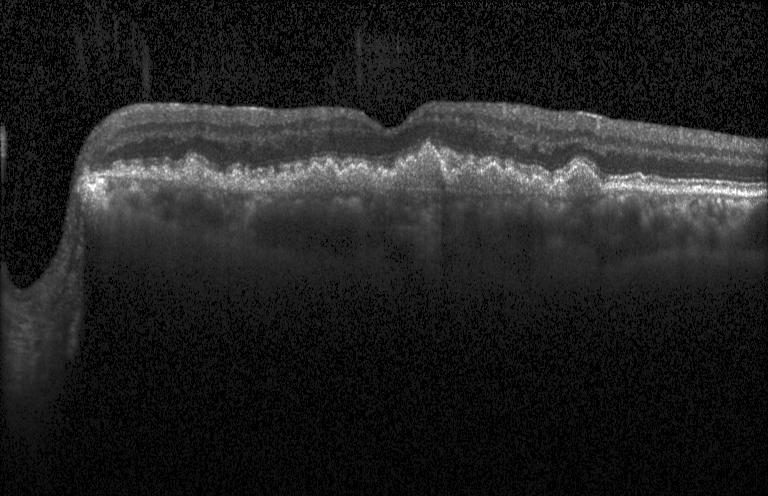

SD-OCT. Retinal OCT B-scan. Centered on the fovea. This B-scan demonstrates choroidal neovascularization.